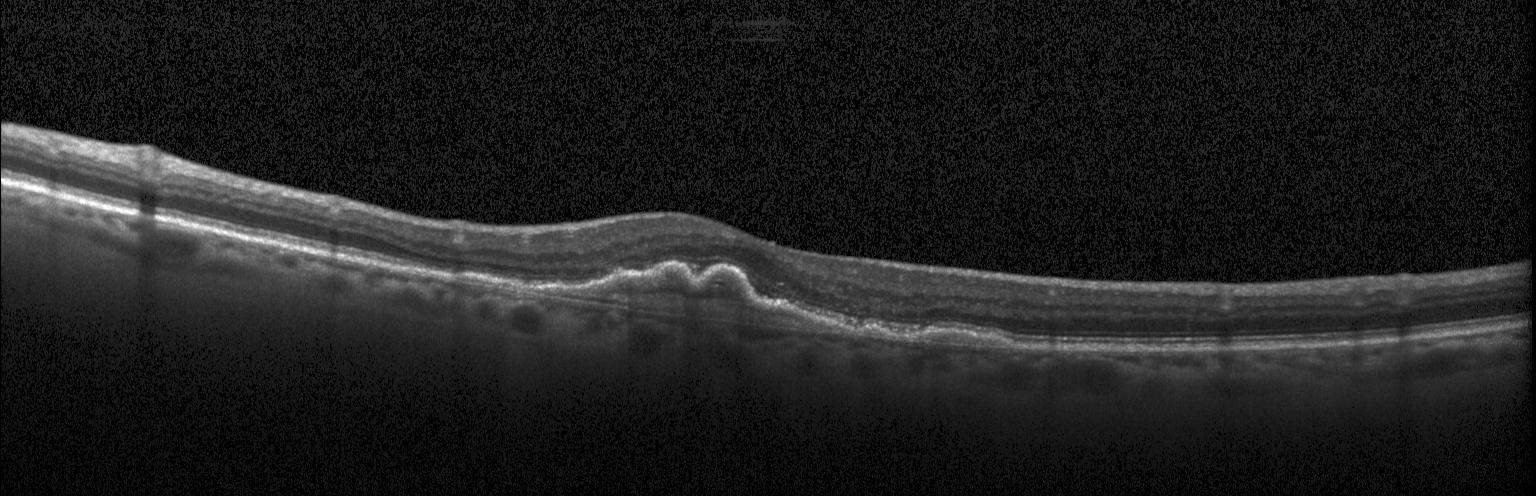 Retinal OCT B-scan.
Impression: choroidal neovascularization (CNV).